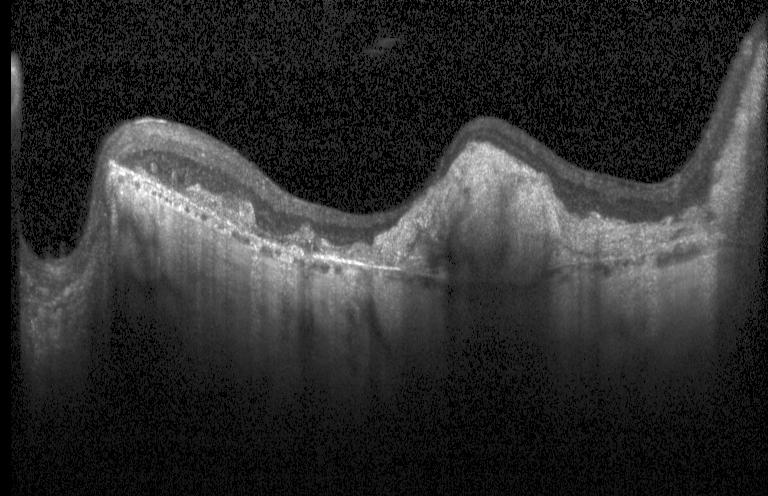
SD-OCT, macular scan, OCT line scan, Heidelberg Spectralis.
Finding: choroidal neovascularization.